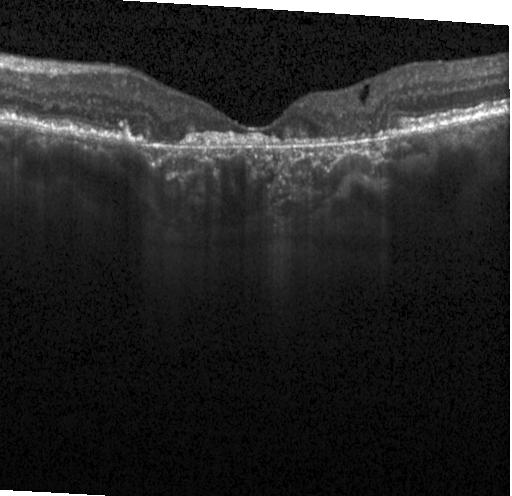

Retinal OCT cross-section · SD-OCT · instrument: Heidelberg Spectralis · horizontal scan through the fovea.
Finding: a choroidal neovascular membrane.